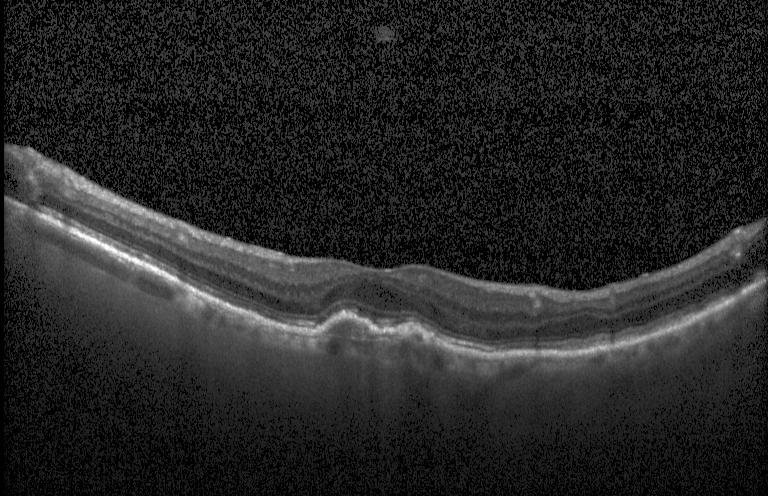 OCT B-scan showing a choroidal neovascular membrane.